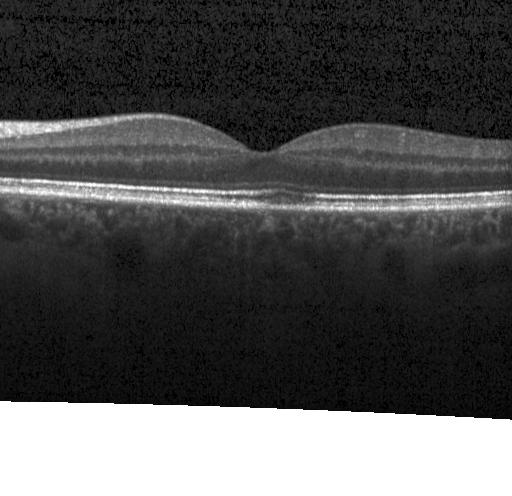 Dx: neither CNV, DME, nor drusen.